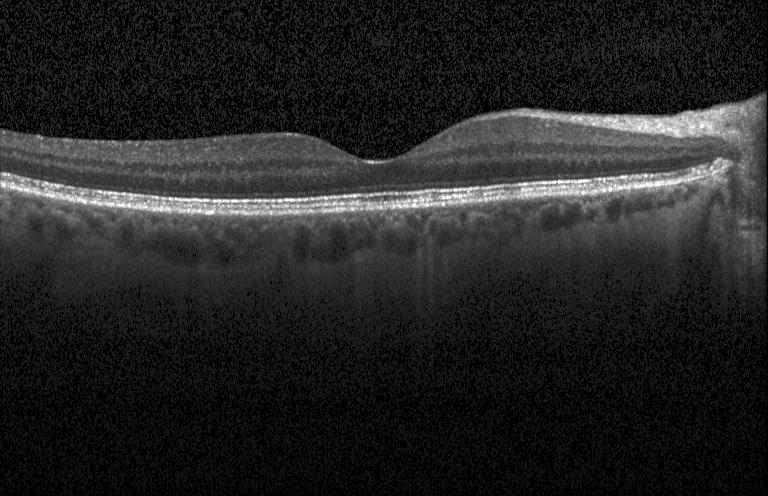

Centered on the fovea, SD-OCT, optical coherence tomography scan, instrument: Heidelberg Spectralis — Finding: no evidence of choroidal neovascularization, diabetic macular edema, or drusen.